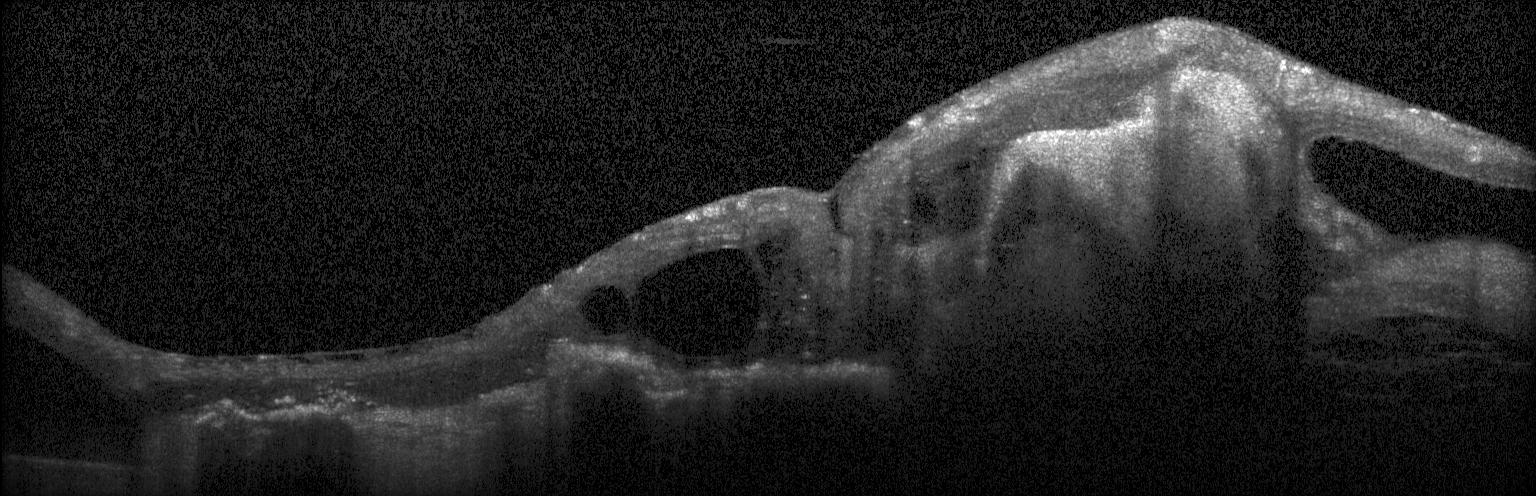
Spectral-domain OCT B-scan: a choroidal neovascular membrane.